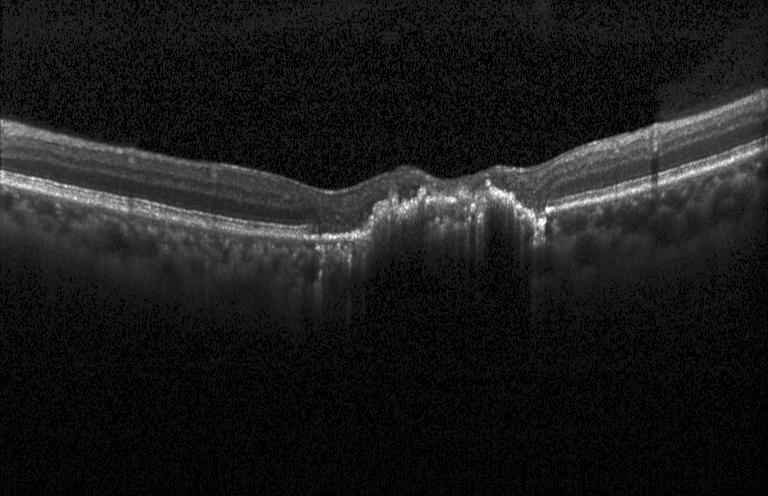
Diagnosis: a choroidal neovascular membrane.